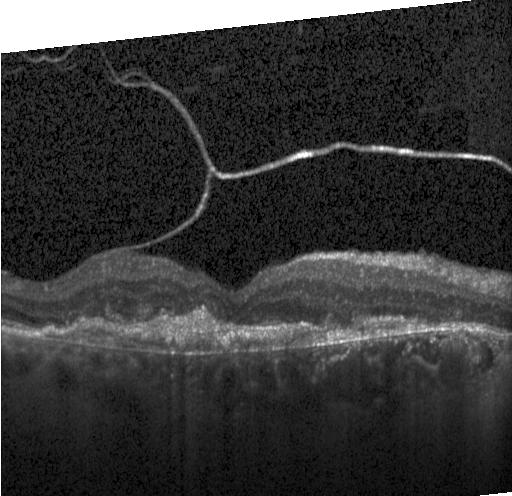 Retinal OCT cross-section.
Dx: CNV.